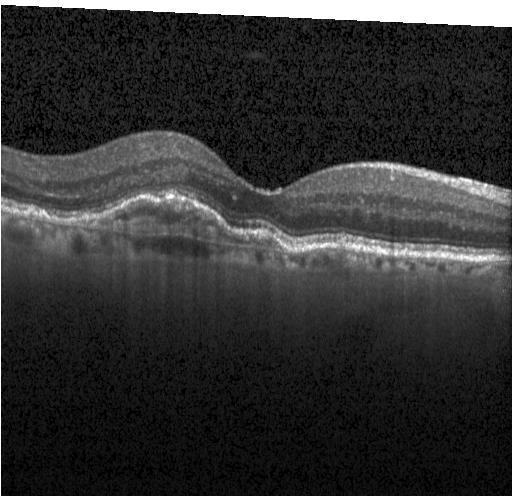 Optical coherence tomography scan, acquired on a Heidelberg Spectralis, centered on the fovea, spectral-domain optical coherence tomography.
Assessment: choroidal neovascularization (CNV).